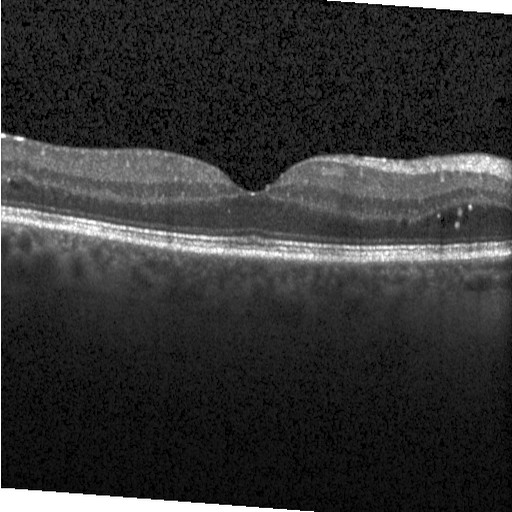
This B-scan demonstrates diabetic macular edema.